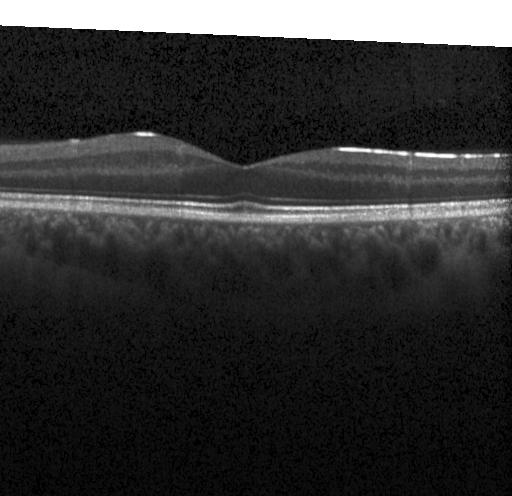 Diagnosis: no evidence of CNV, DME, or drusen.